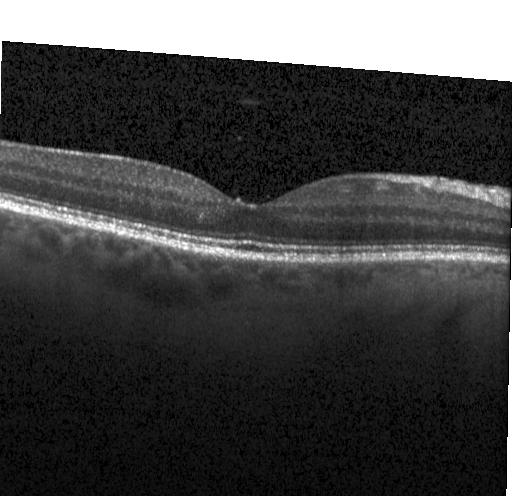 Impression: no choroidal neovascularization, no diabetic macular edema, and no drusen.